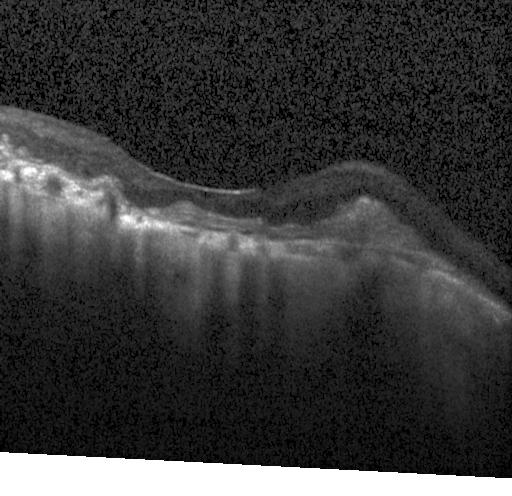
Retinal OCT cross-section
The scan shows a choroidal neovascular membrane.